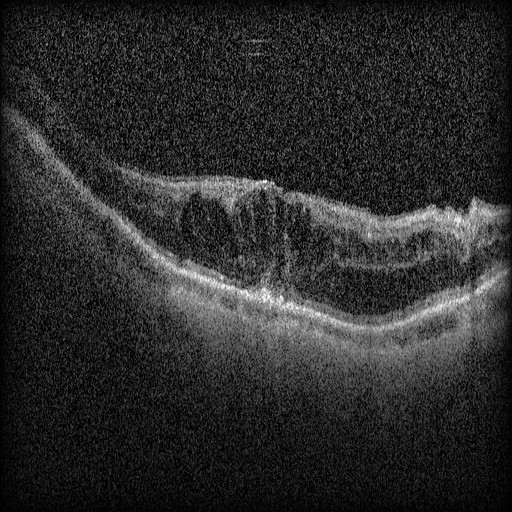
Dx: diabetic macular edema.